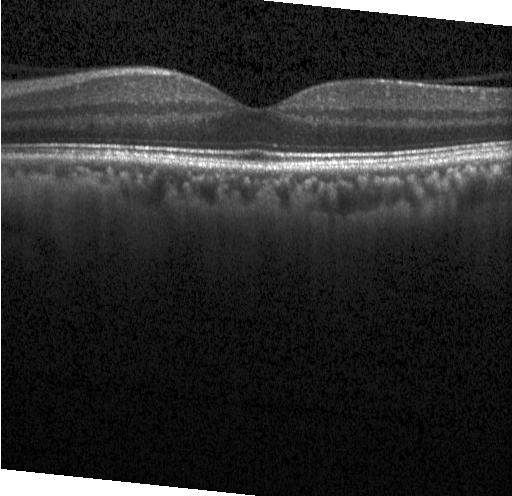
Spectral-domain OCT. Horizontal scan through the fovea. Acquired on a Heidelberg Spectralis. OCT B-scan
Dx: no choroidal neovascularization, no diabetic macular edema, and no drusen.